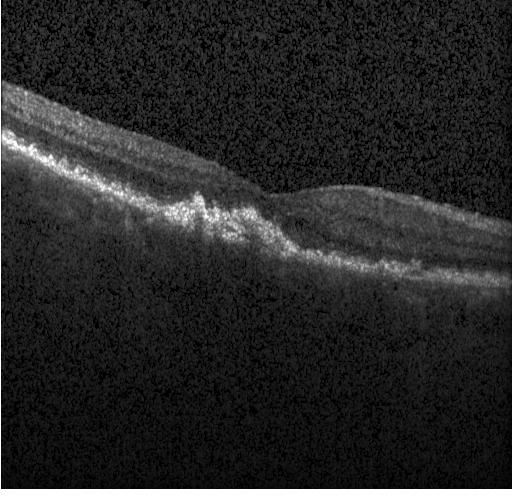

Optical coherence tomography scan; Heidelberg Spectralis OCT system; spectral-domain optical coherence tomography — The scan shows choroidal neovascularization (CNV).